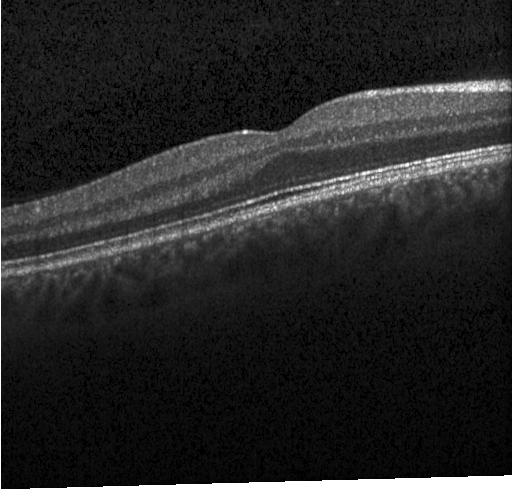
Optical coherence tomography B-scan — OCT finding: no choroidal neovascularization, no diabetic macular edema, and no drusen.